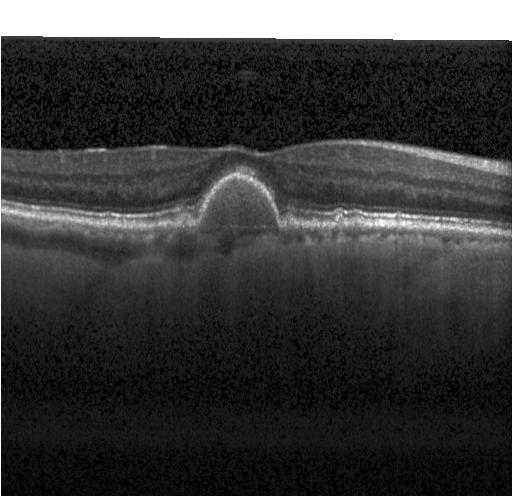
Retinal OCT cross-section.
The scan shows a choroidal neovascular membrane.